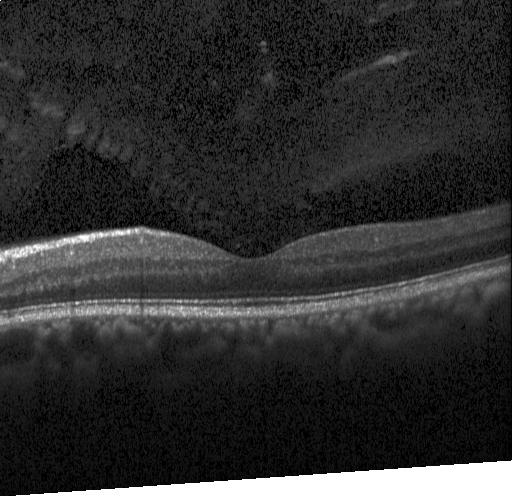

Fovea-centered; spectral-domain OCT; OCT line scan.
This B-scan demonstrates no evidence of choroidal neovascularization, diabetic macular edema, or drusen.